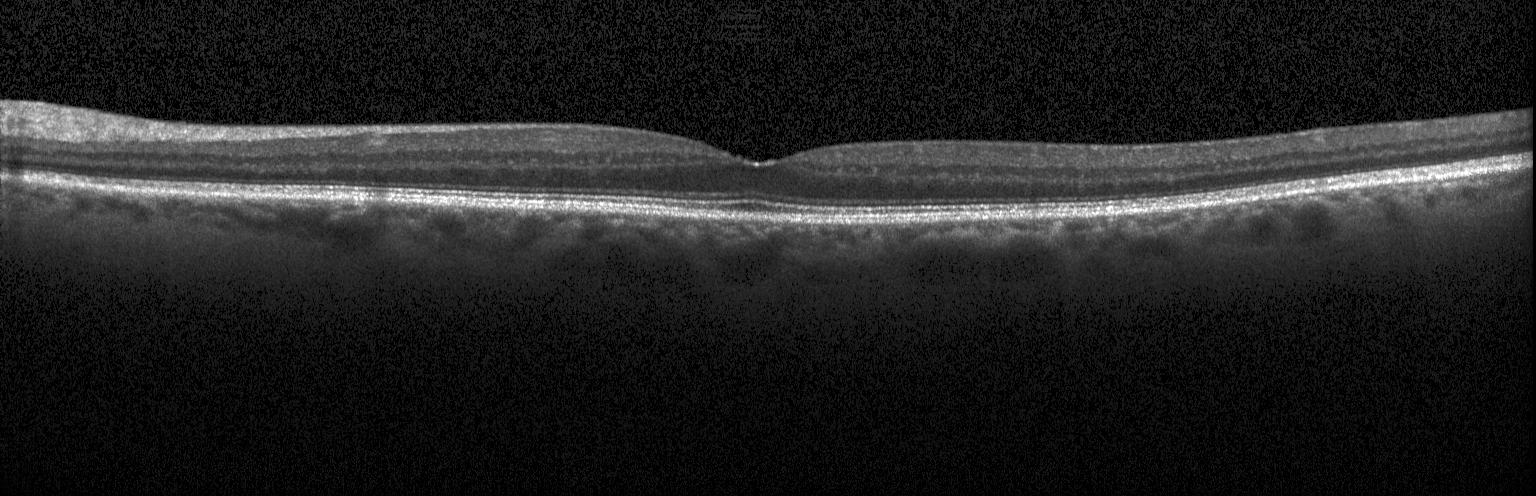

Assessment: no choroidal neovascularization, no diabetic macular edema, and no drusen.